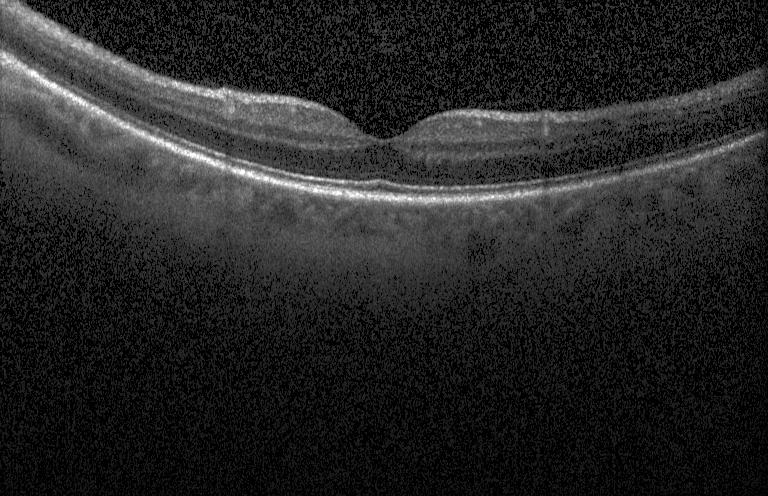

Dx: neither choroidal neovascularization, diabetic macular edema, nor drusen.